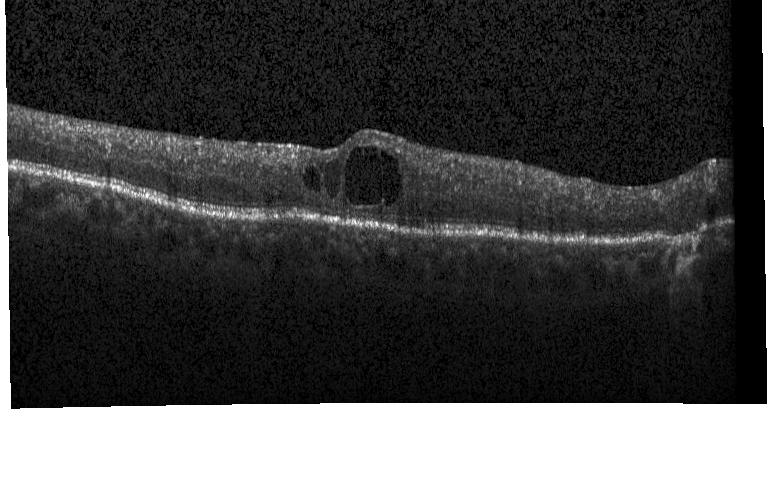 Macular scan. OCT line scan. Heidelberg Spectralis OCT system
Macular OCT: diabetic macular edema.